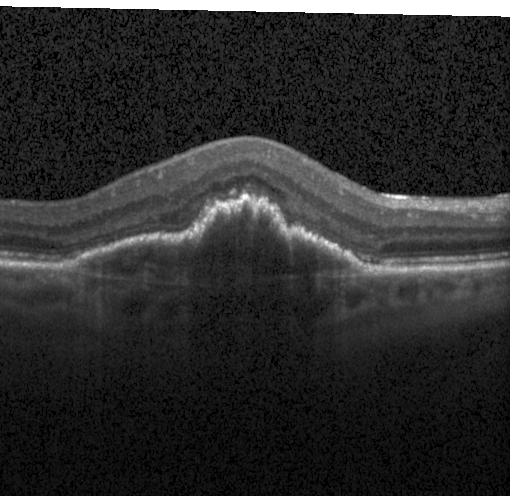
OCT B-scan — The scan shows choroidal neovascularization (CNV).